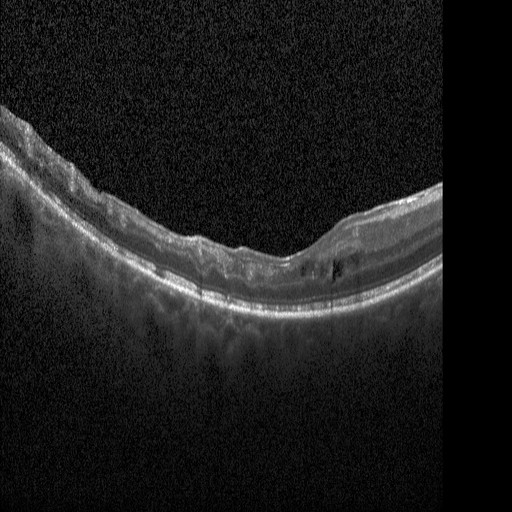 Retinal OCT B-scan.
The scan shows DME.